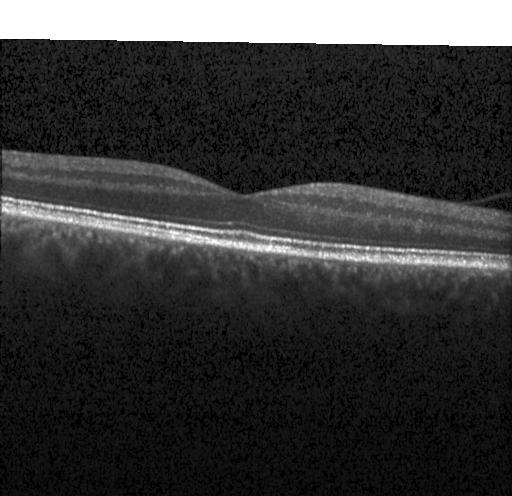 OCT scan showing no choroidal neovascularization, diabetic macular edema, or drusen.